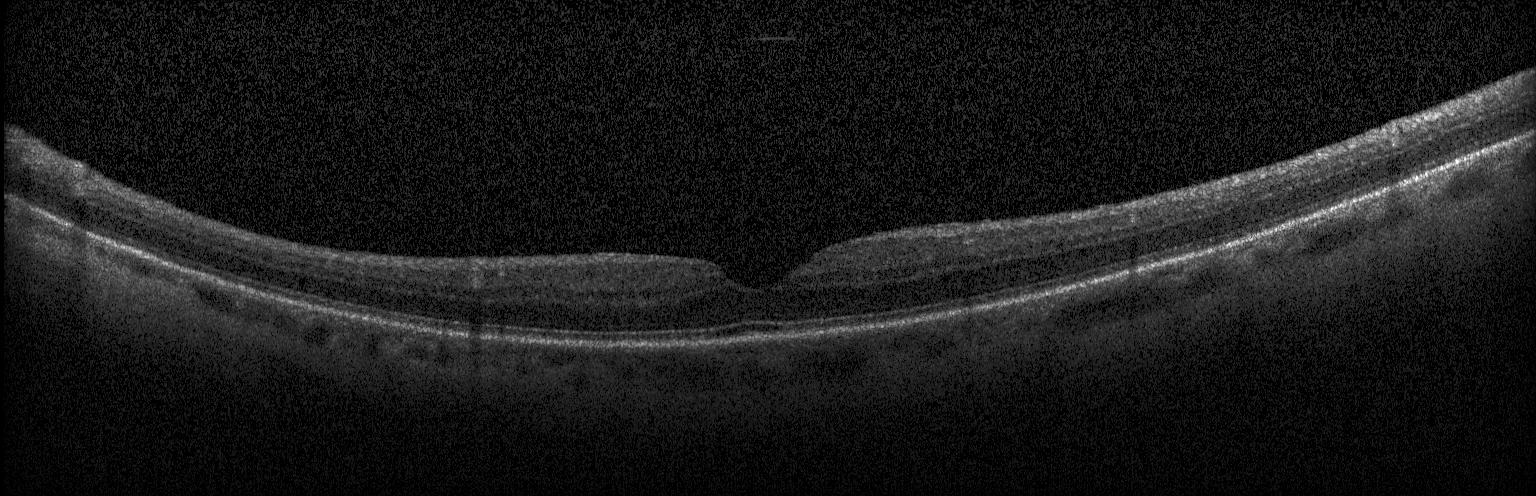 Optical coherence tomography B-scan · horizontal scan through the fovea · instrument: Heidelberg Spectralis · spectral-domain optical coherence tomography. Impression: no choroidal neovascularization, no diabetic macular edema, and no drusen.